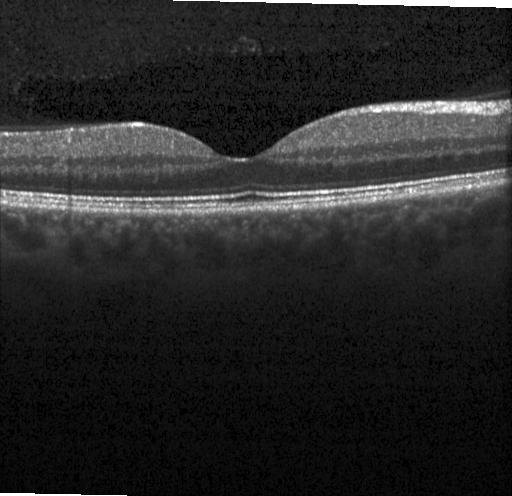

Retinal OCT B-scan, Heidelberg Spectralis.
Assessment: no evidence of choroidal neovascularization, diabetic macular edema, or drusen.